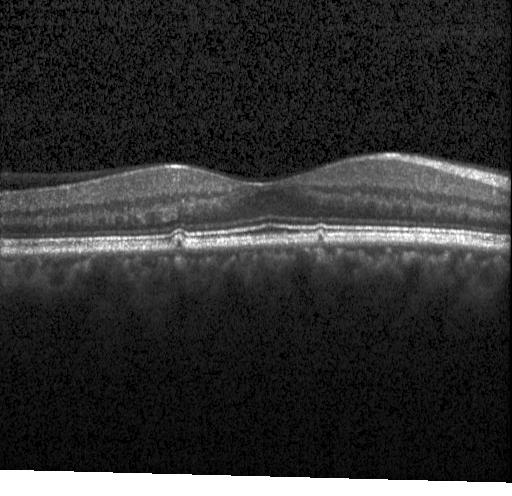
This B-scan demonstrates sub-RPE drusenoid deposits.